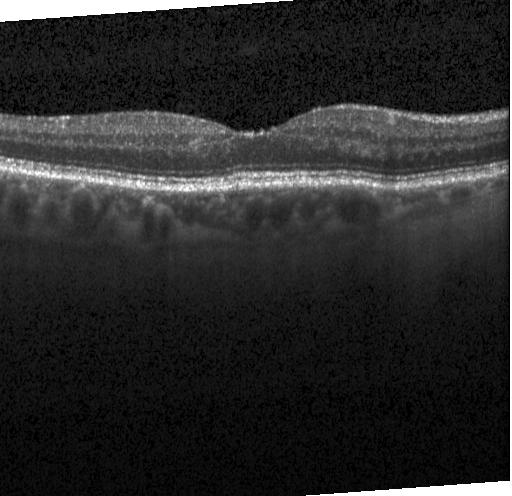 Dx: no evidence of choroidal neovascularization, diabetic macular edema, or drusen.